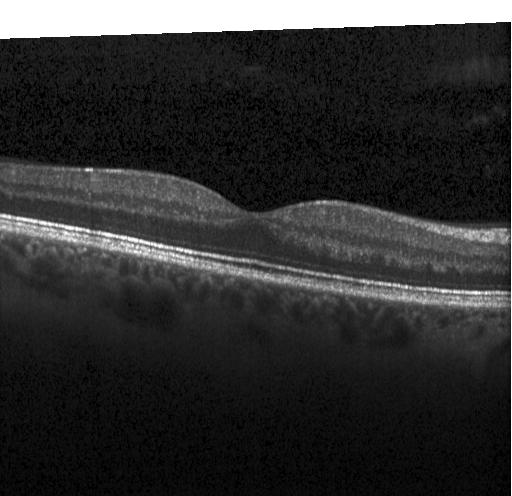 Retinal OCT cross-section · horizontal scan through the fovea
Impression: no choroidal neovascularization, diabetic macular edema, or drusen.